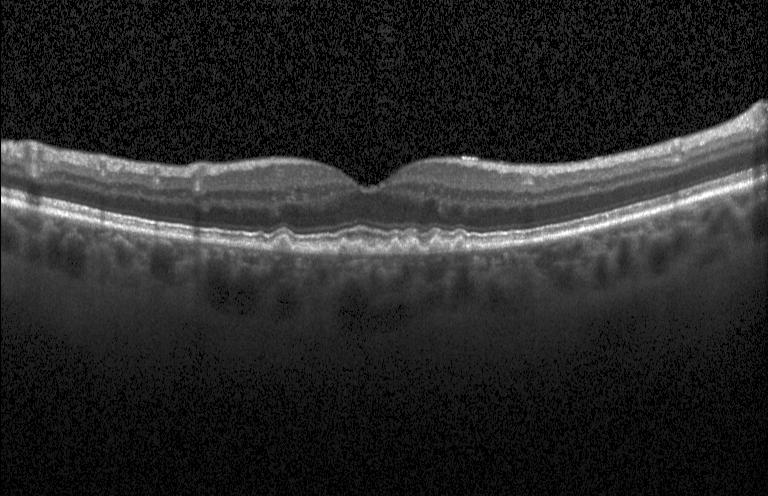

Optical coherence tomography scan. Heidelberg Spectralis OCT system. This B-scan demonstrates sub-RPE drusenoid deposits.